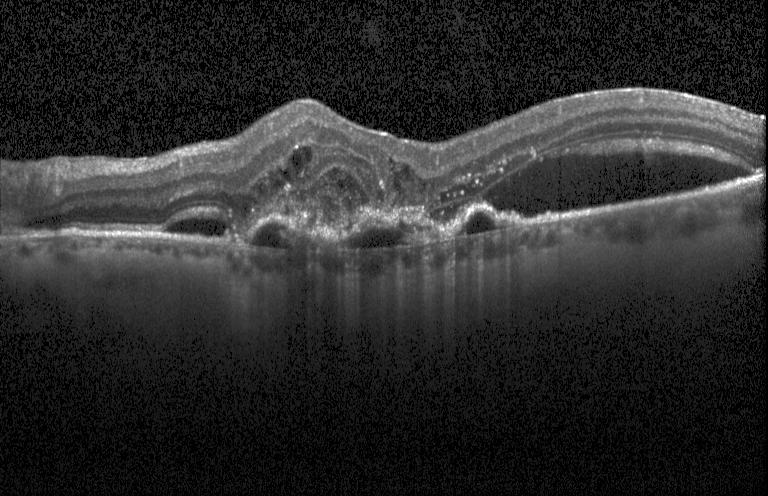

SD-OCT; retinal OCT B-scan; instrument: Heidelberg Spectralis — Macular OCT: CNV.